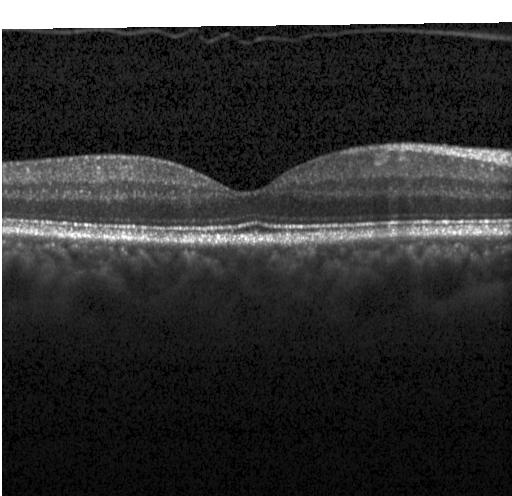

Diagnosis: no choroidal neovascularization, no diabetic macular edema, and no drusen.